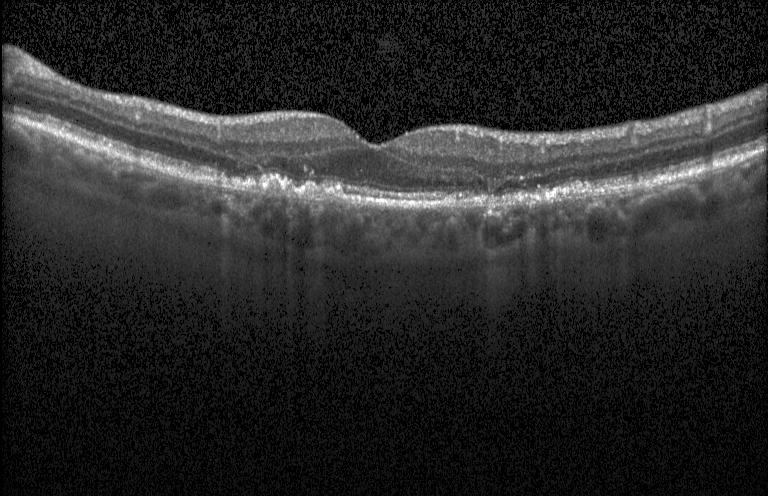 Diagnosis: sub-RPE drusenoid deposits.